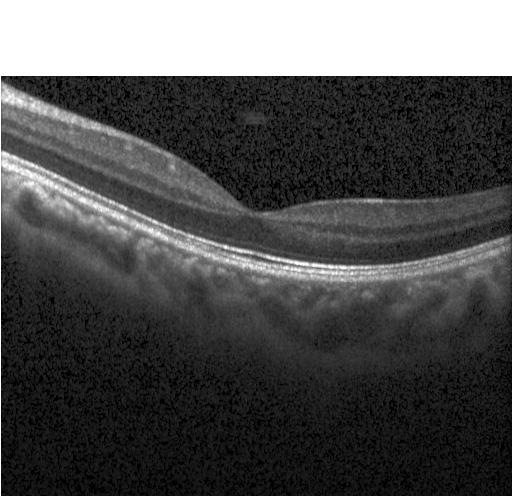
Heidelberg Spectralis, retinal OCT B-scan.
This B-scan demonstrates no choroidal neovascularization, no diabetic macular edema, and no drusen.